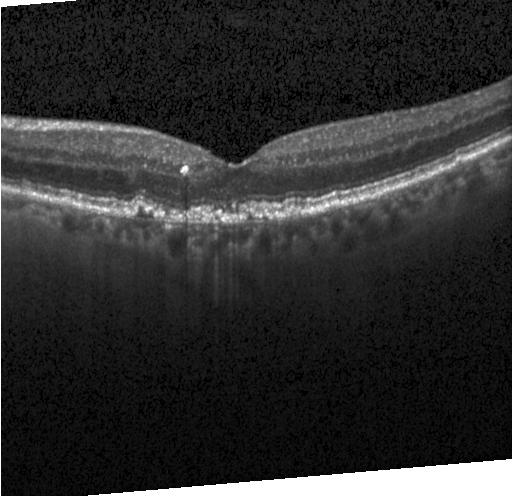
Impression: a choroidal neovascular membrane.